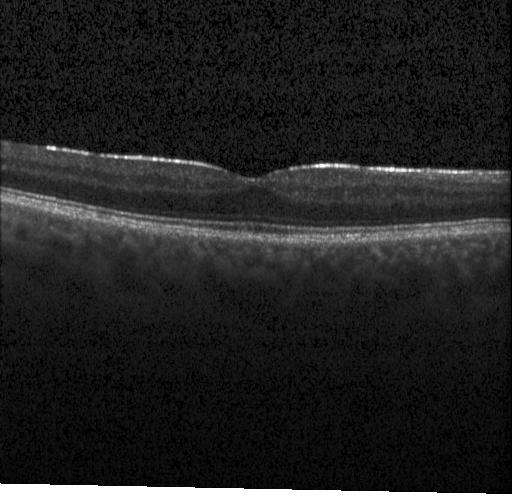 OCT finding: no choroidal neovascularization, diabetic macular edema, or drusen.